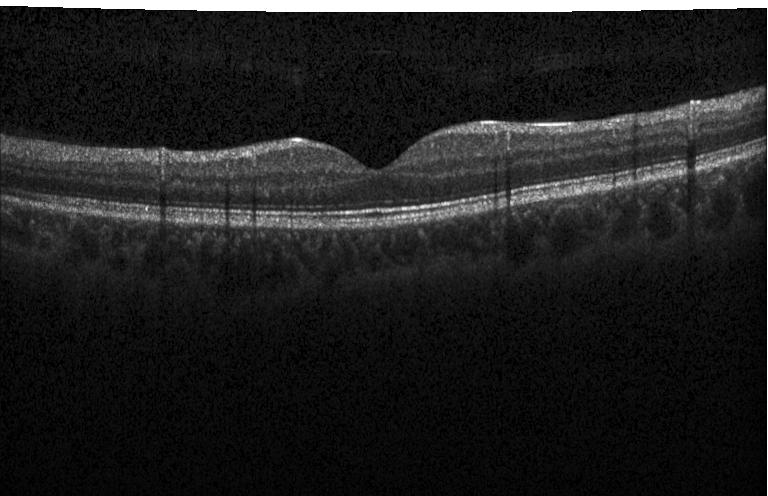
Optical coherence tomography scan · instrument: Heidelberg Spectralis · spectral-domain optical coherence tomography. Neither choroidal neovascularization, diabetic macular edema, nor drusen.